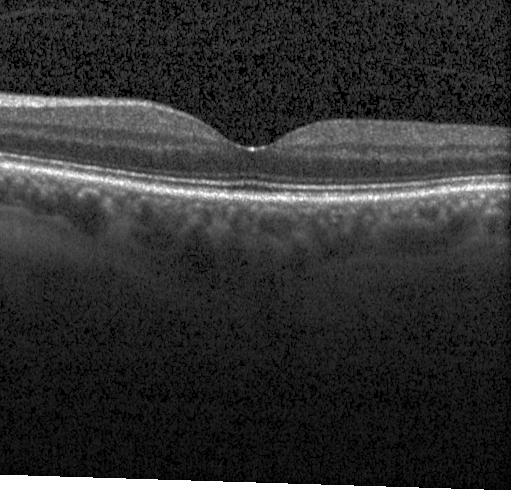

Dx: no choroidal neovascularization, no diabetic macular edema, and no drusen.